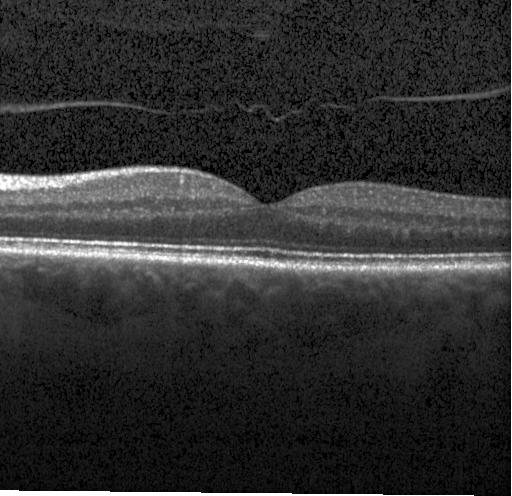
Macular scan; spectral-domain OCT; retinal OCT cross-section
Macular OCT: no CNV, DME, or drusen.